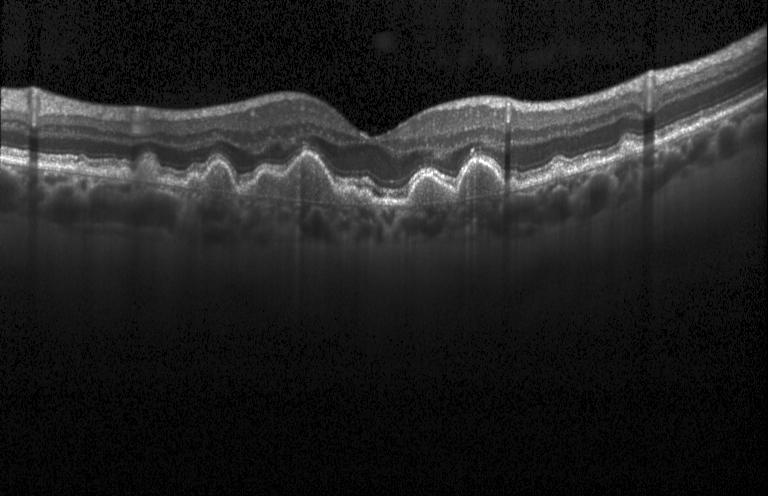
Drusen.